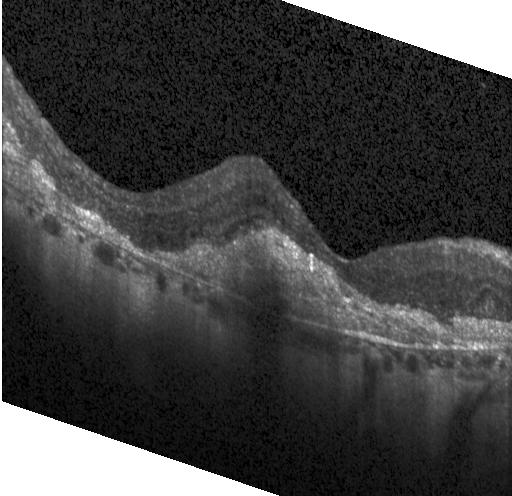

Finding: a choroidal neovascular membrane.